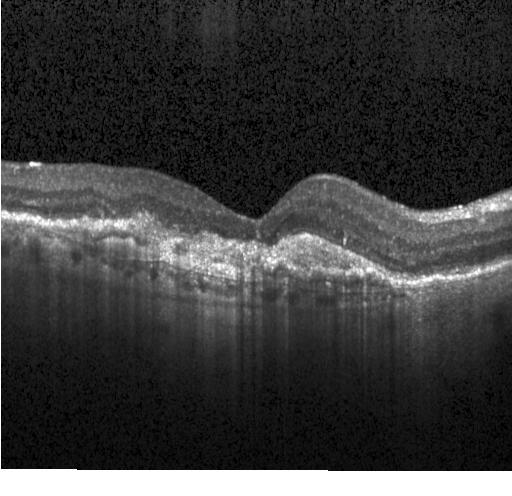 Heidelberg Spectralis OCT system · optical coherence tomography B-scan · centered on the fovea — This B-scan demonstrates CNV.